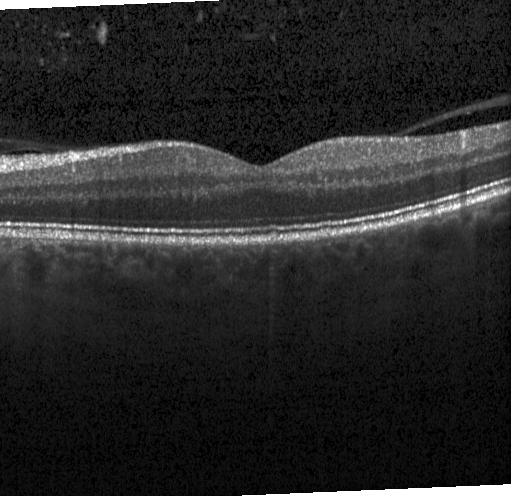

Spectral-domain OCT; horizontal scan through the fovea; optical coherence tomography B-scan
Finding: neither CNV, DME, nor drusen.